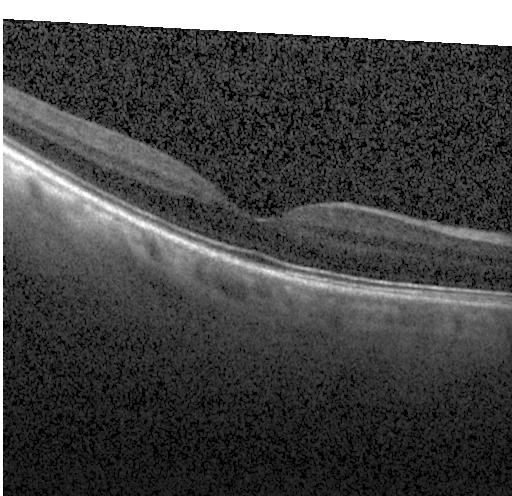

No CNV, DME, or drusen.